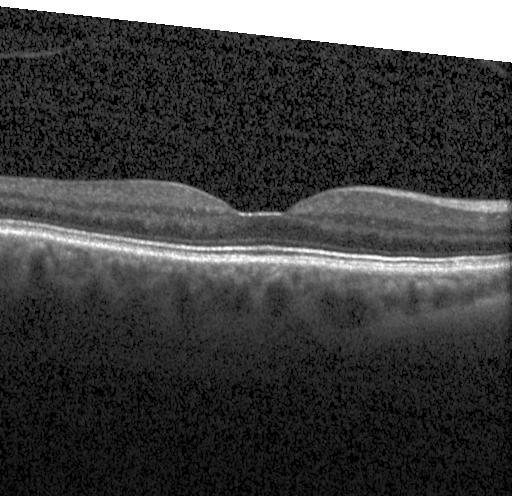

OCT finding: neither choroidal neovascularization, diabetic macular edema, nor drusen.